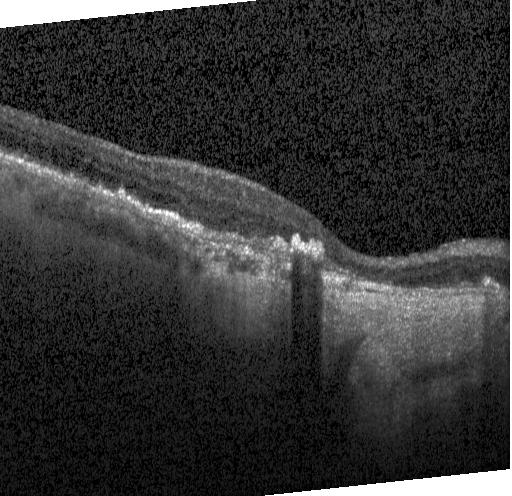

Optical coherence tomography B-scan
This B-scan demonstrates a choroidal neovascular membrane.